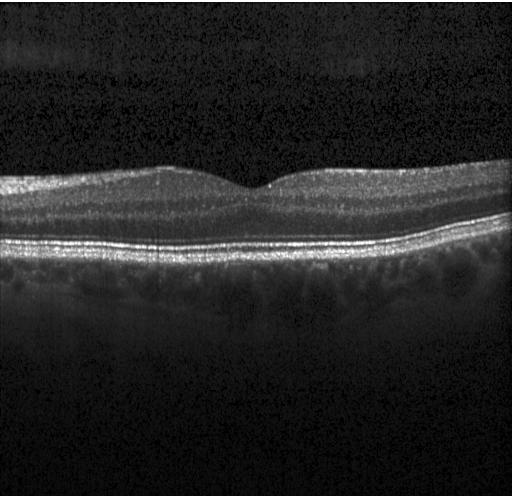

OCT B-scan. Diagnosis: no CNV, no DME, and no drusen.